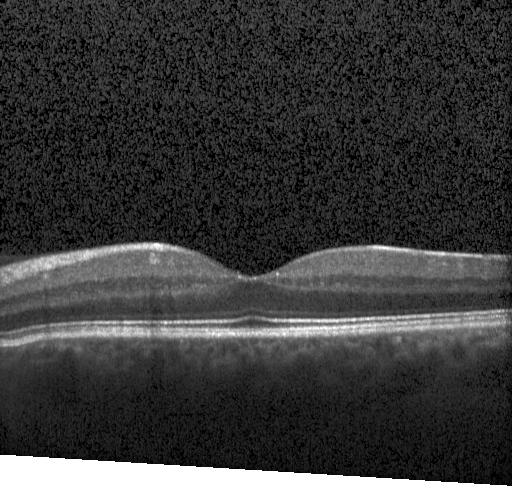

Finding: no choroidal neovascularization, no diabetic macular edema, and no drusen.